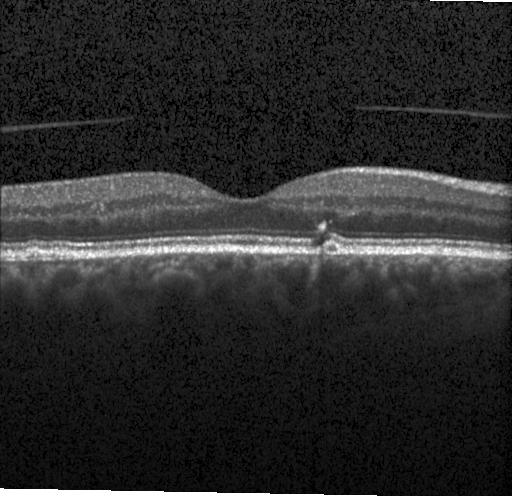 OCT B-scan, SD-OCT.
Assessment: multiple drusen.